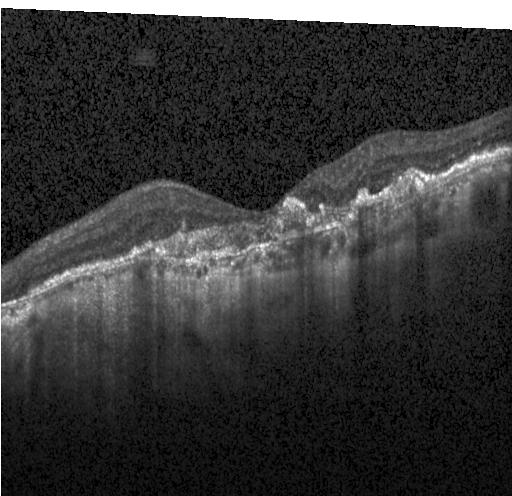 Retinal OCT B-scan, horizontal scan through the fovea, spectral-domain optical coherence tomography.
Finding: choroidal neovascularization (CNV).